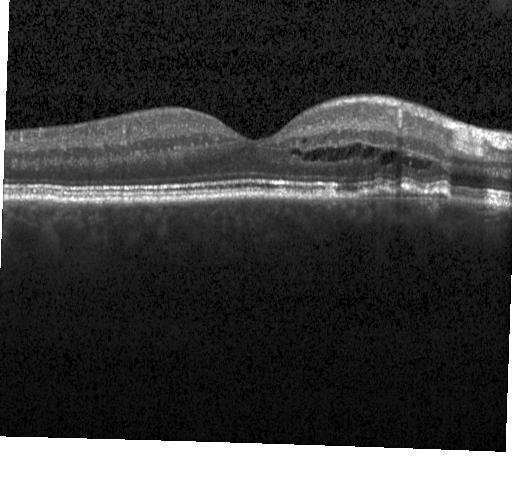 Macular OCT demonstrating a choroidal neovascular membrane.